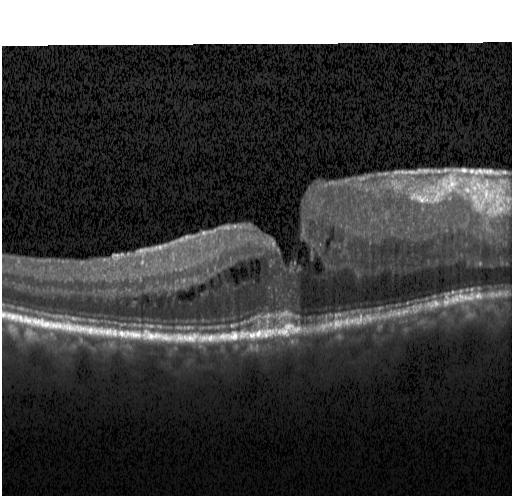
OCT scan showing DME.